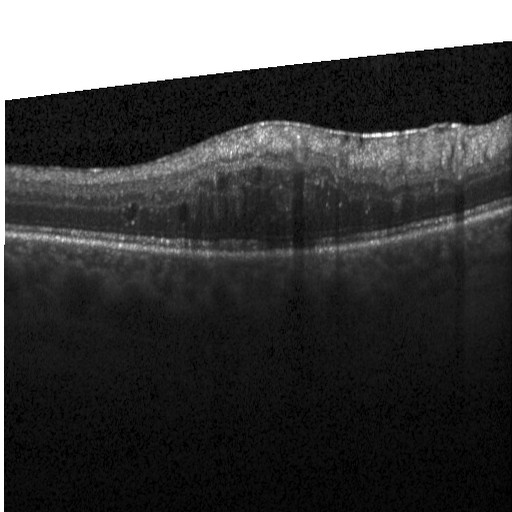 Diagnosis: diabetic macular edema.